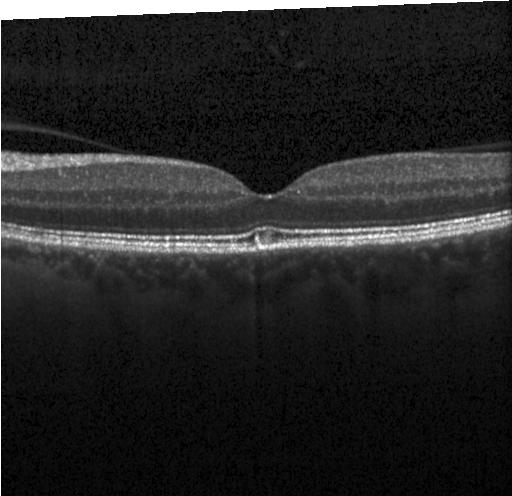
Impression: no CNV, no DME, and no drusen.